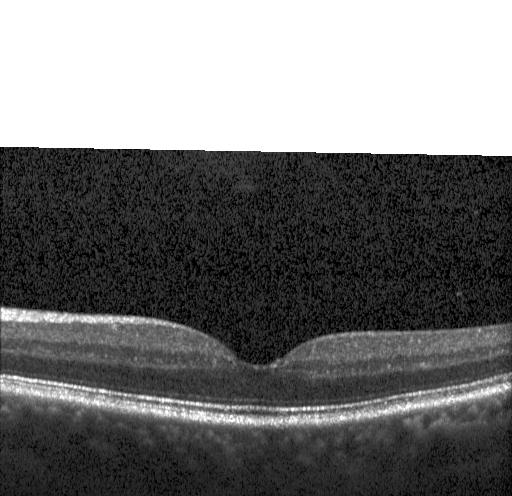
Instrument: Heidelberg Spectralis. OCT B-scan — Neither choroidal neovascularization, diabetic macular edema, nor drusen.